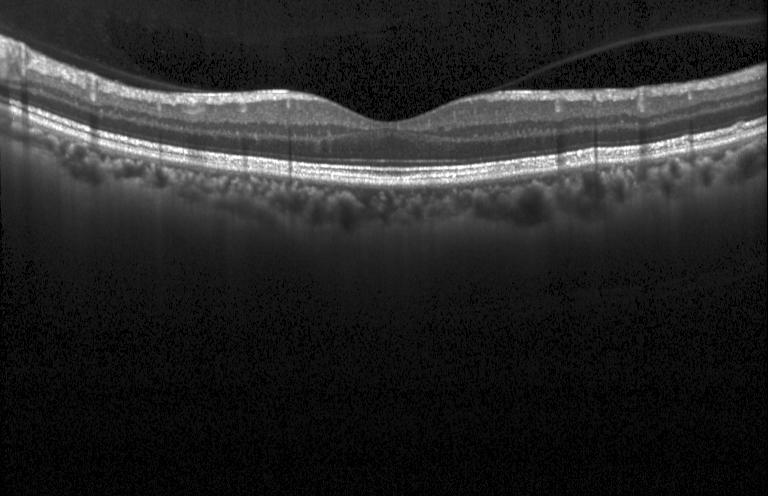 The scan shows neither CNV, DME, nor drusen.